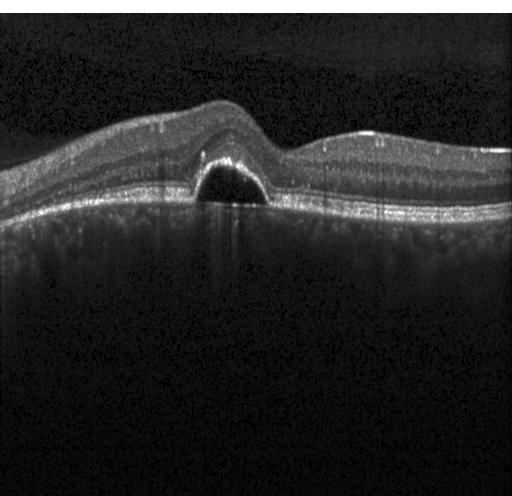
Diagnosis: CNV.